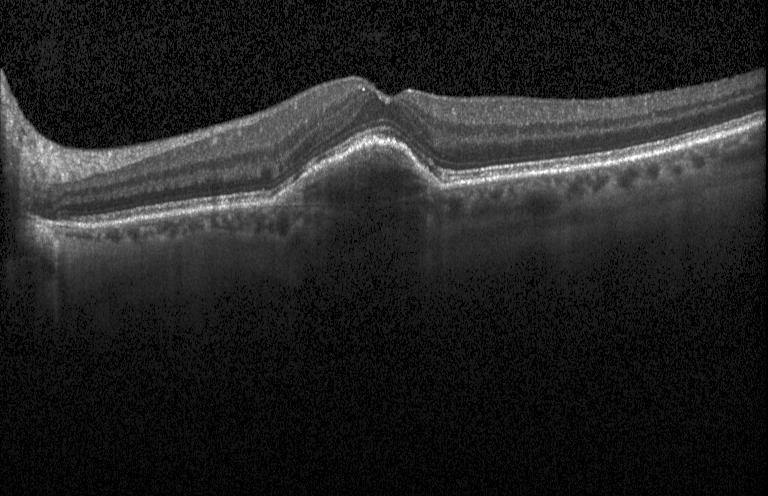 OCT line scan — Diagnosis: a choroidal neovascular membrane.